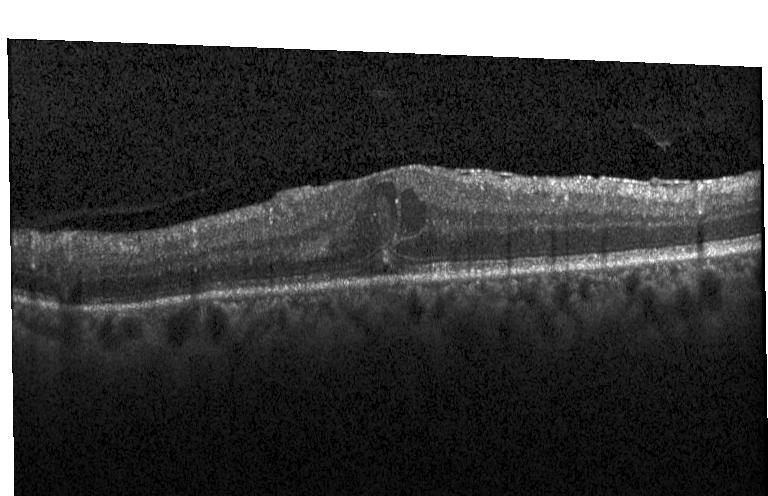 OCT line scan — Diagnosis: DME.